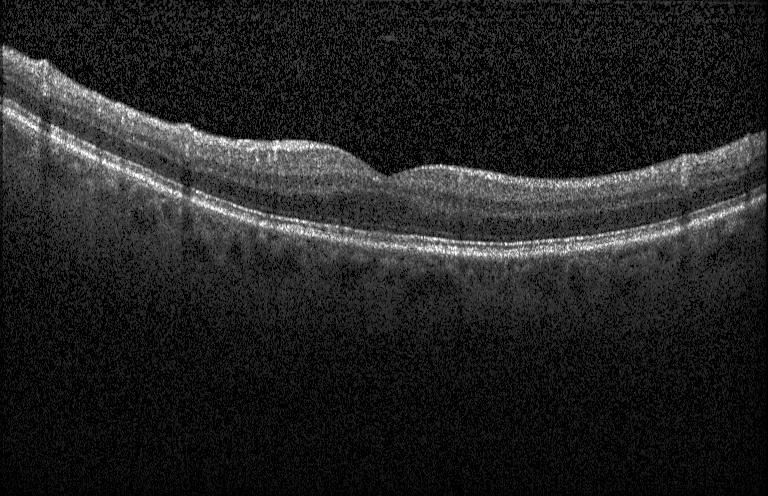

Retinal OCT B-scan
Finding: no evidence of CNV, DME, or drusen.